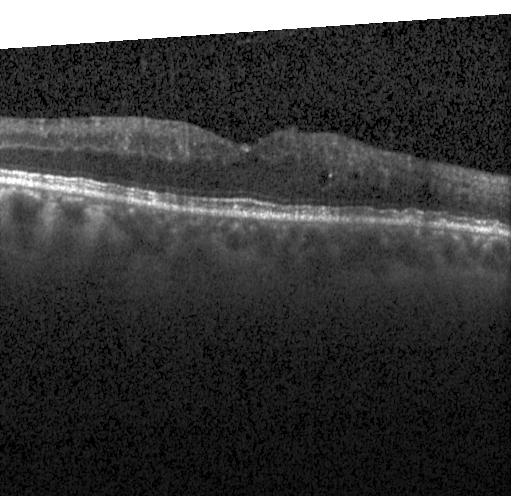

Impression: diabetic macular edema.